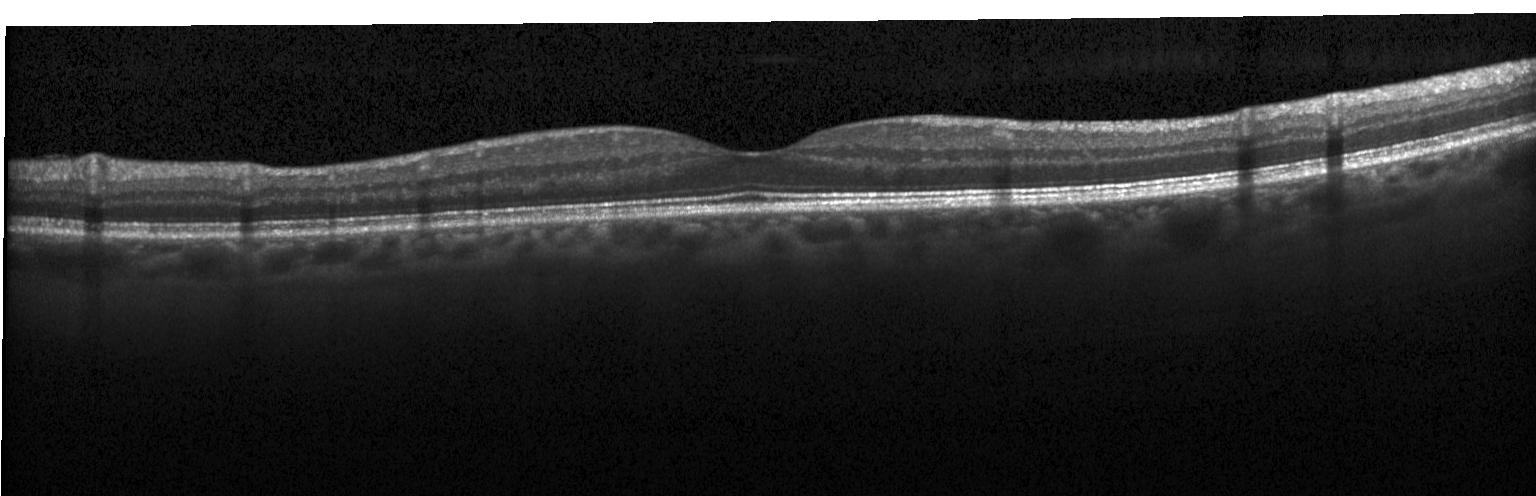 Heidelberg Spectralis OCT system · retinal OCT cross-section. This B-scan demonstrates no evidence of choroidal neovascularization, diabetic macular edema, or drusen.